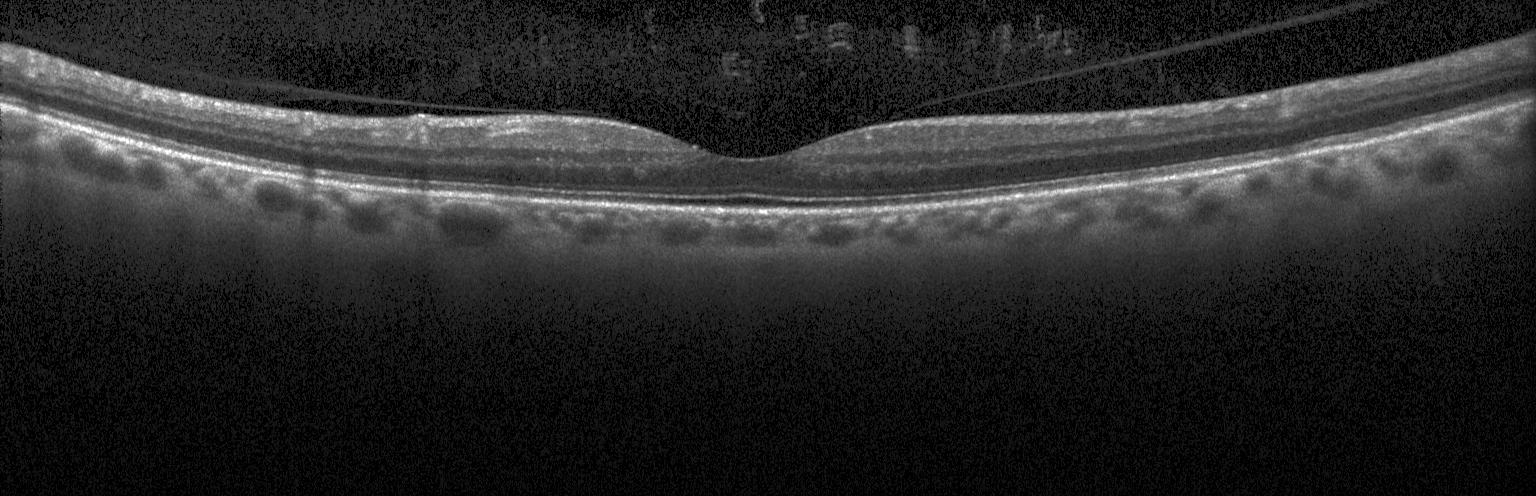

Finding: no evidence of CNV, DME, or drusen.